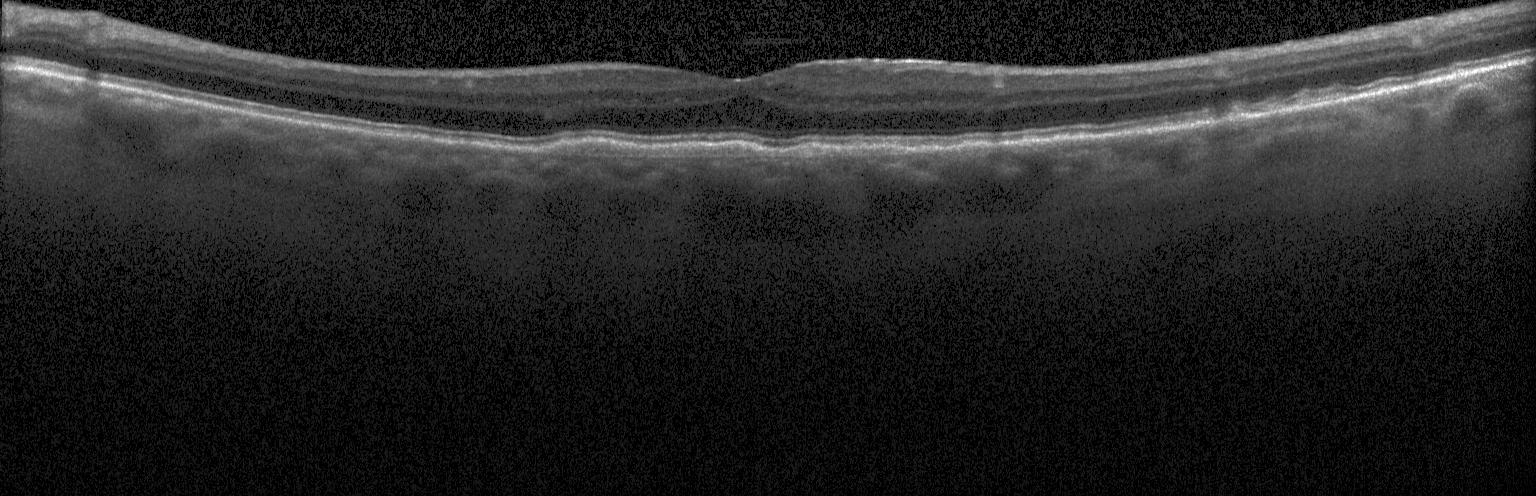

Dx: choroidal neovascularization (CNV).